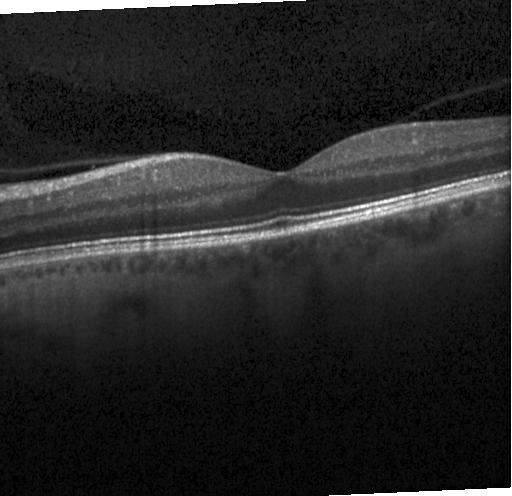
Optical coherence tomography scan; spectral-domain optical coherence tomography; centered on the fovea; Heidelberg Spectralis — Impression: no choroidal neovascularization, diabetic macular edema, or drusen.